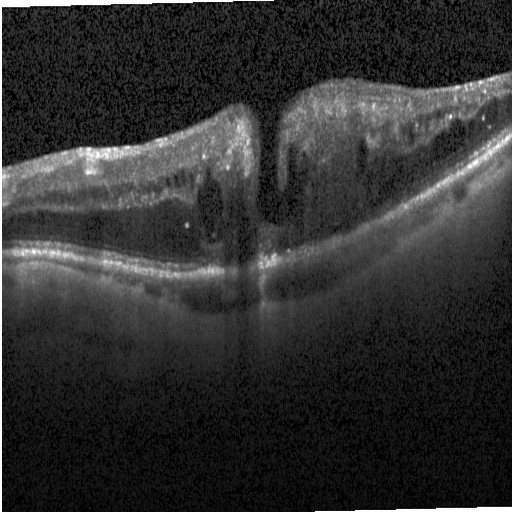
OCT B-scan. Macular scan. Acquired on a Heidelberg Spectralis
Finding: diabetic macular edema (DME).